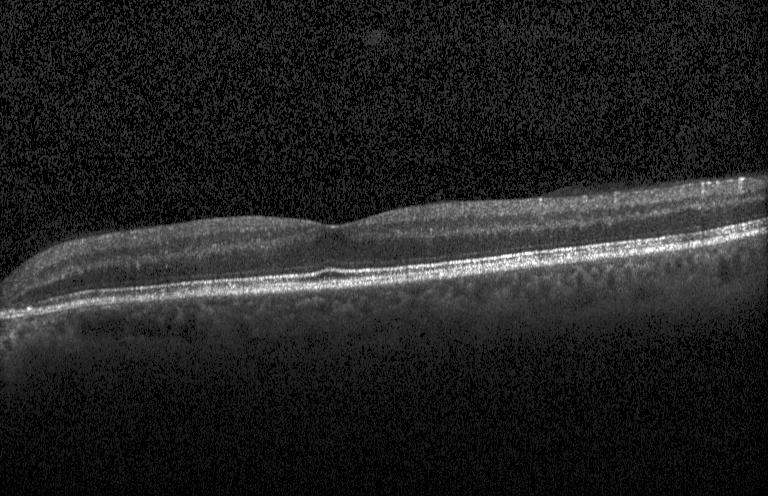

Dx: no evidence of choroidal neovascularization, diabetic macular edema, or drusen.